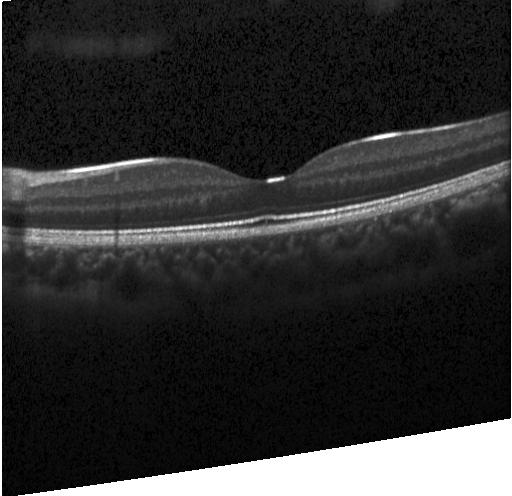

SD-OCT; retinal OCT cross-section — Assessment: no choroidal neovascularization, no diabetic macular edema, and no drusen.